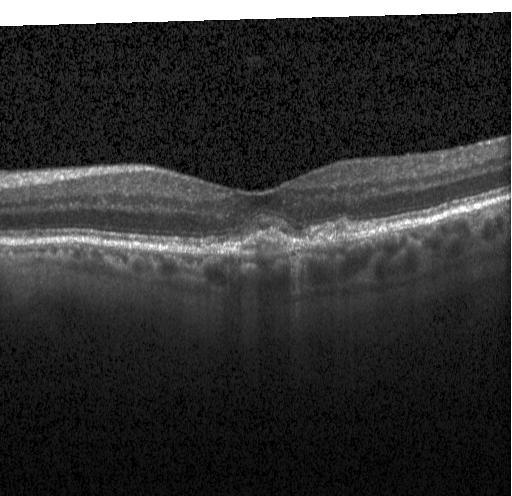

Acquired on a Heidelberg Spectralis; centered on the fovea; optical coherence tomography scan; SD-OCT
Diagnosis: a choroidal neovascular membrane.